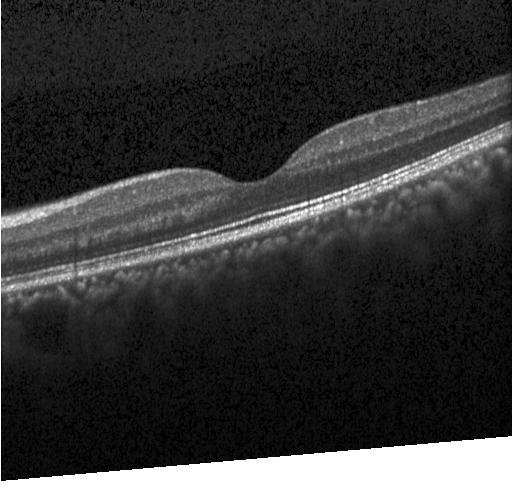

Optical coherence tomography scan. No CNV, DME, or drusen.